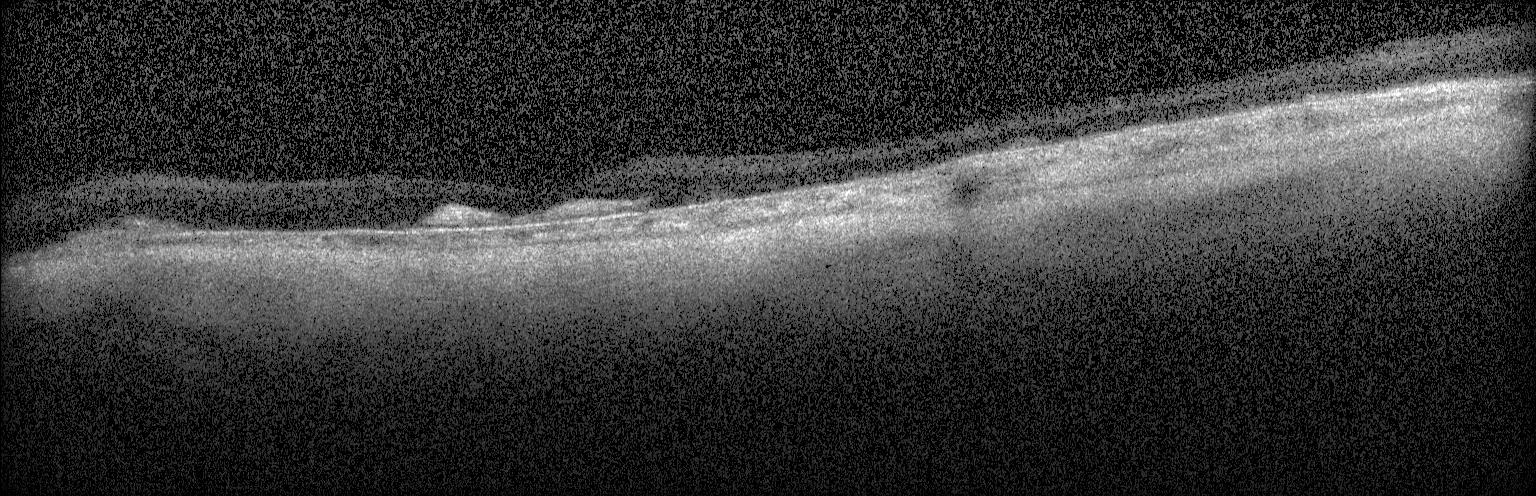
Heidelberg Spectralis OCT system; OCT line scan; spectral-domain optical coherence tomography
OCT finding: a choroidal neovascular membrane.